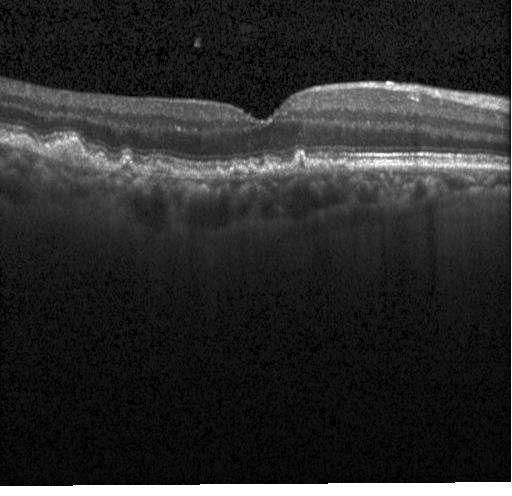

OCT scan showing sub-RPE drusenoid deposits.